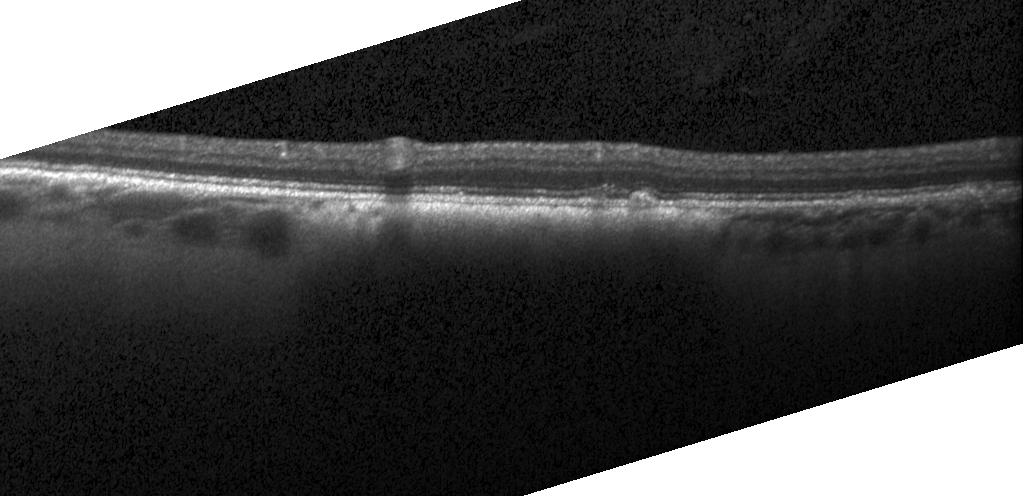 Retinal OCT cross-section · spectral-domain OCT · acquired on a Heidelberg Spectralis · fovea-centered
Finding: a choroidal neovascular membrane.